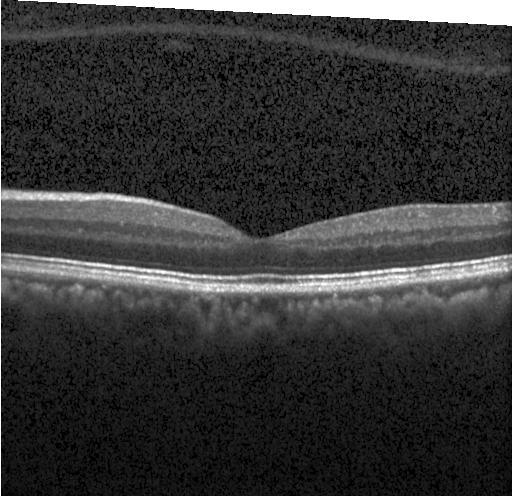 OCT finding: neither CNV, DME, nor drusen.